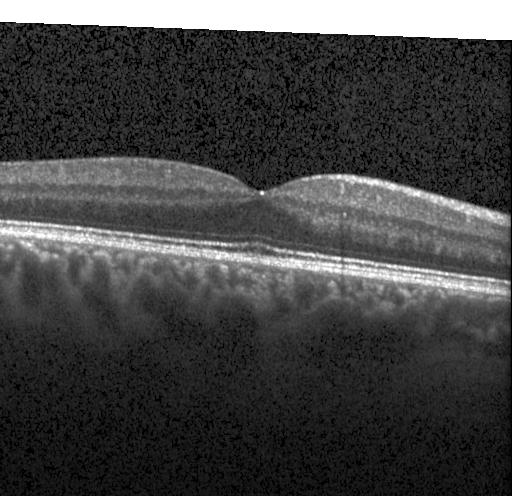 Retinal OCT cross-section, centered on the fovea, Heidelberg Spectralis, spectral-domain optical coherence tomography
This B-scan demonstrates no CNV, no DME, and no drusen.